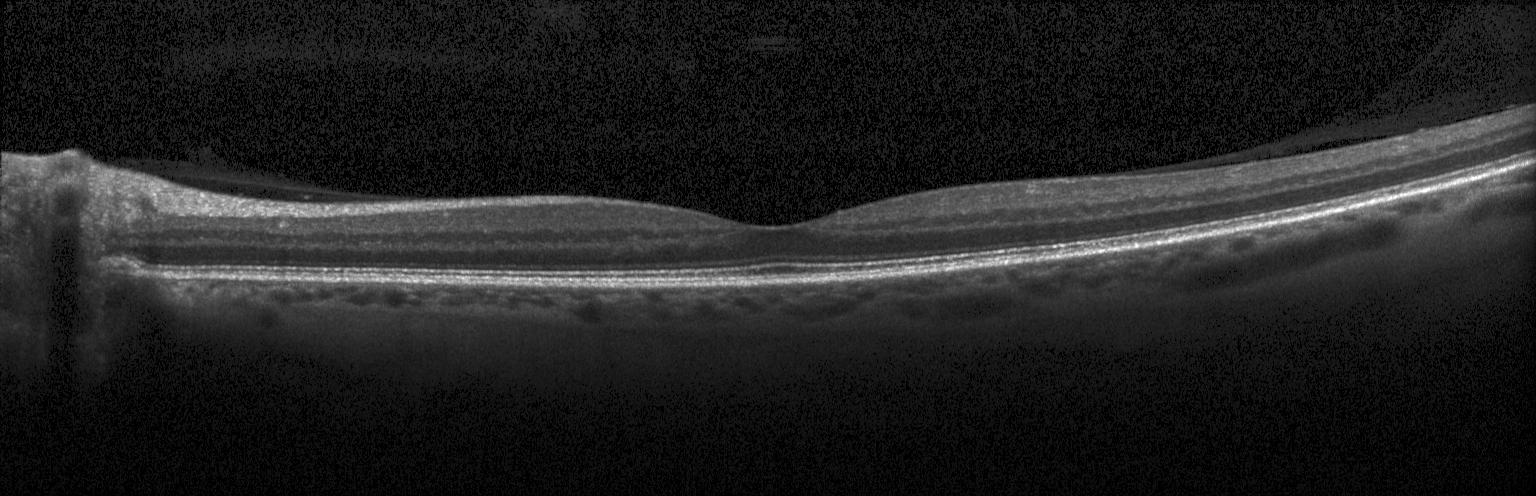

OCT finding: no choroidal neovascularization, no diabetic macular edema, and no drusen.